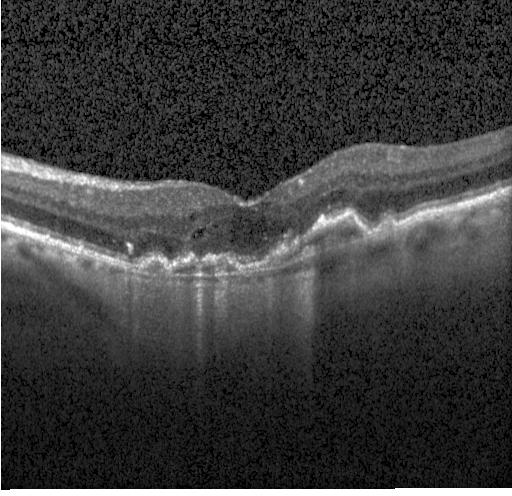 SD-OCT, optical coherence tomography scan, instrument: Heidelberg Spectralis. The scan shows CNV.